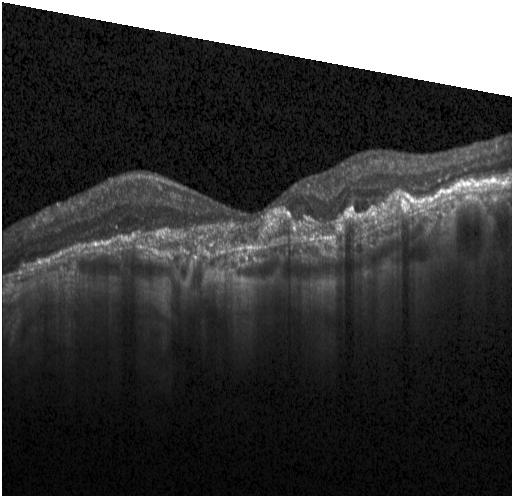
Impression: choroidal neovascularization (CNV).